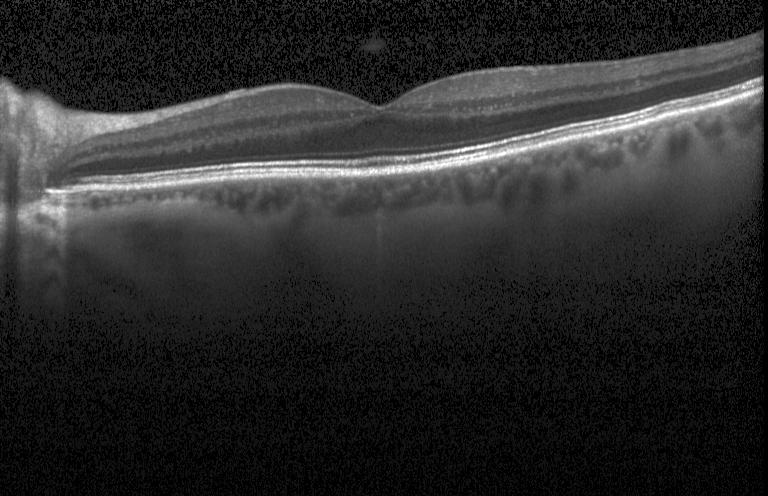 OCT finding: neither choroidal neovascularization, diabetic macular edema, nor drusen.